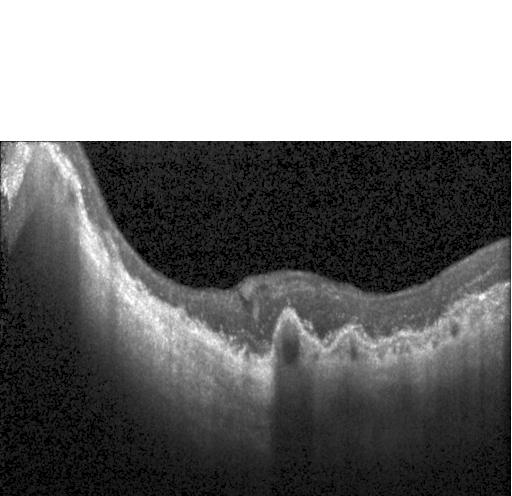 Optical coherence tomography scan, horizontal scan through the fovea, Heidelberg Spectralis. The scan shows choroidal neovascularization.